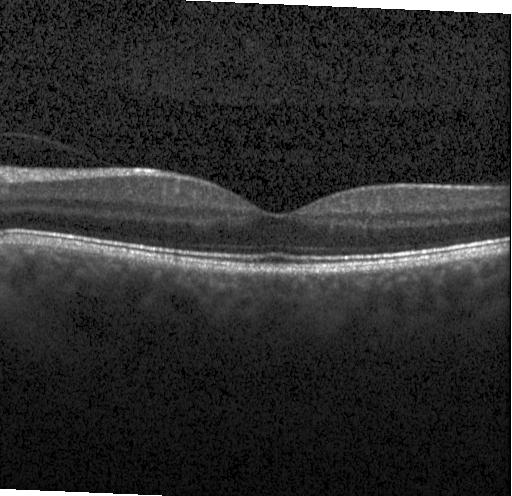 Centered on the fovea; OCT line scan. Impression: no CNV, no DME, and no drusen.